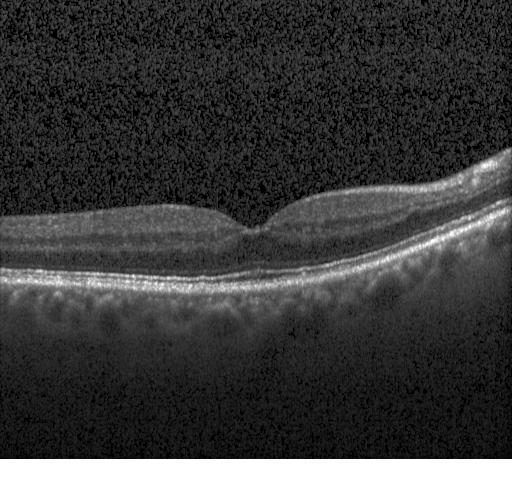

SD-OCT, OCT line scan, acquired on a Heidelberg Spectralis
Macular OCT: no choroidal neovascularization, diabetic macular edema, or drusen.